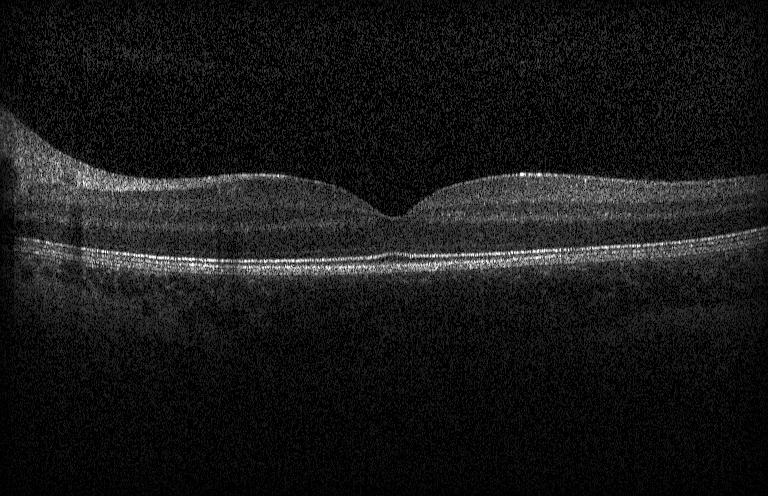 Through the macula, SD-OCT, optical coherence tomography scan, instrument: Heidelberg Spectralis — Finding: neither CNV, DME, nor drusen.